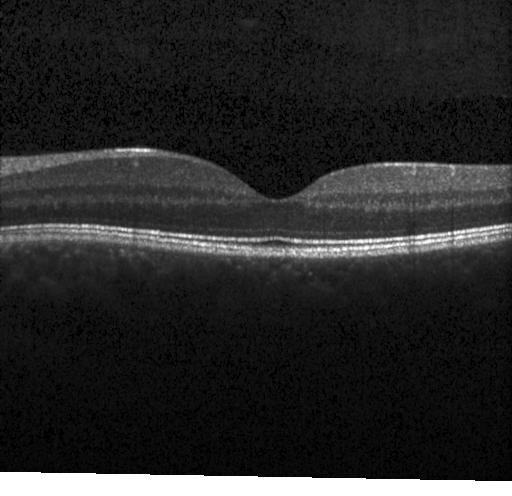

Finding: no evidence of choroidal neovascularization, diabetic macular edema, or drusen.